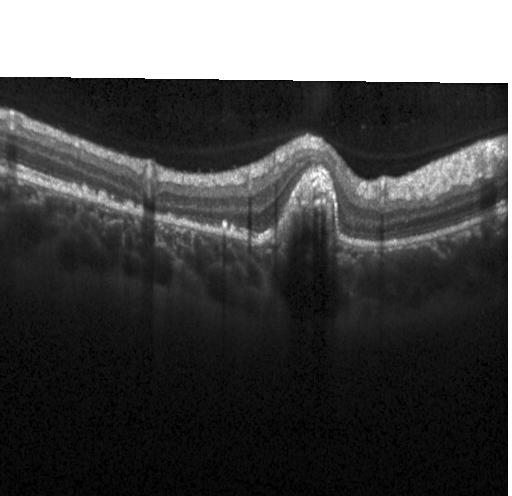
Optical coherence tomography B-scan. Macular OCT: choroidal neovascularization (CNV).